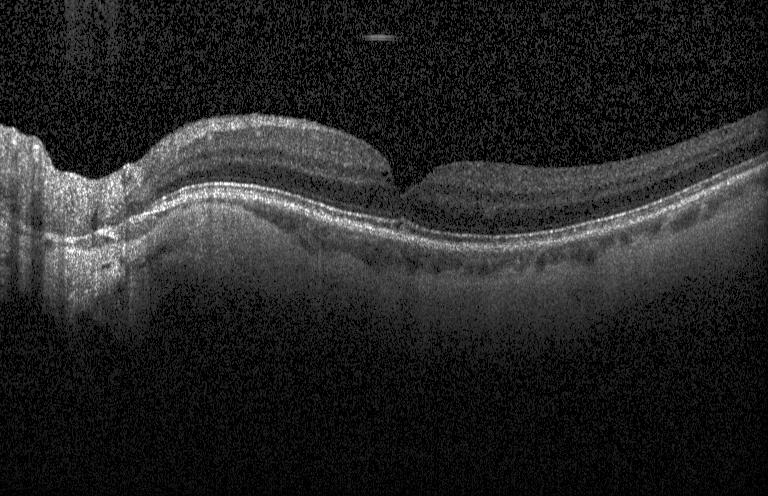 Optical coherence tomography scan. Fovea-centered
Neither choroidal neovascularization, diabetic macular edema, nor drusen.